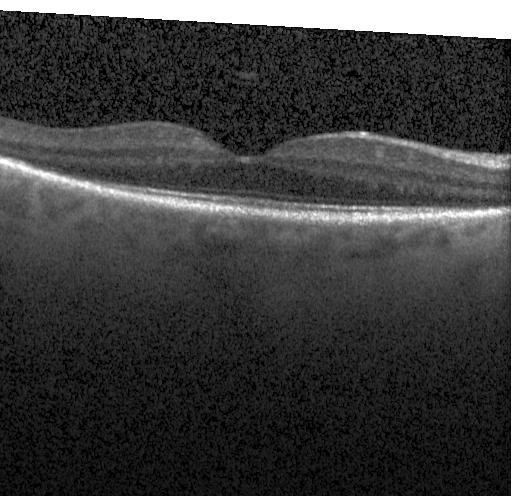 Retinal OCT B-scan · instrument: Heidelberg Spectralis
Diagnosis: neither choroidal neovascularization, diabetic macular edema, nor drusen.